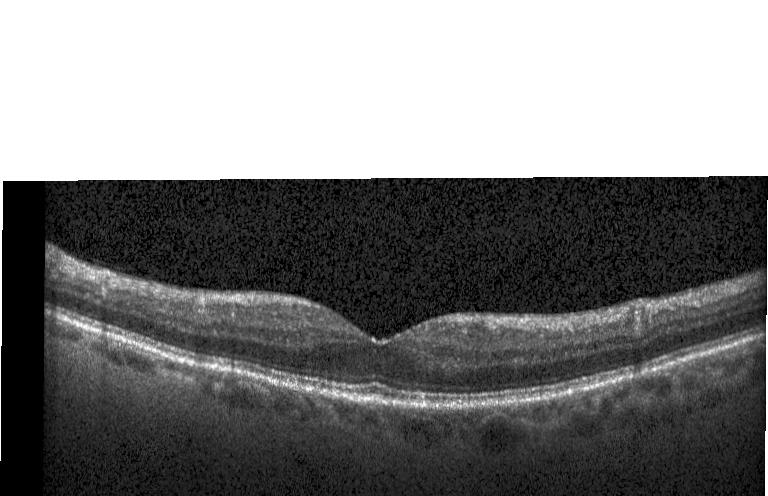 Retinal OCT cross-section showing no choroidal neovascularization, diabetic macular edema, or drusen.